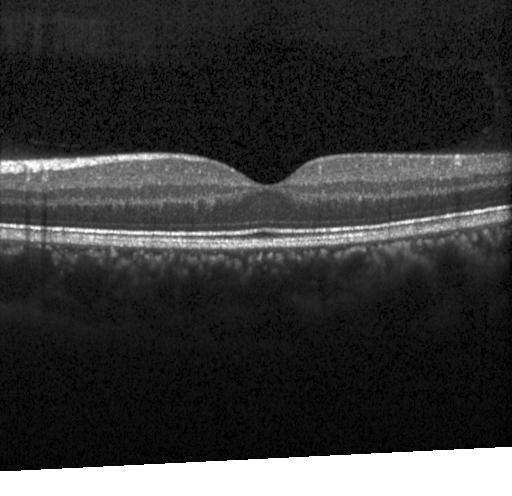

SD-OCT; retinal OCT B-scan; horizontal scan through the fovea; instrument: Heidelberg Spectralis.
Diagnosis: no CNV, DME, or drusen.